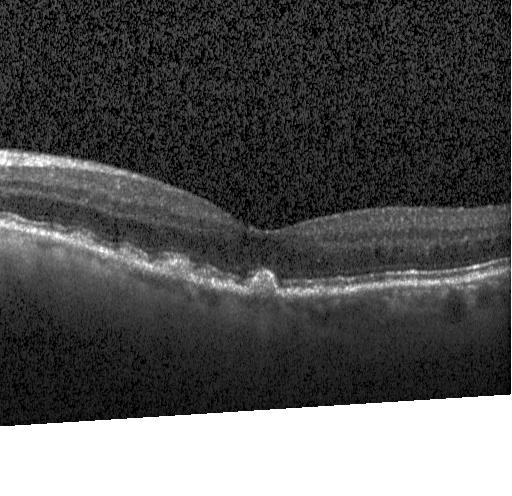
Optical coherence tomography scan.
Diagnosis: sub-RPE drusenoid deposits.